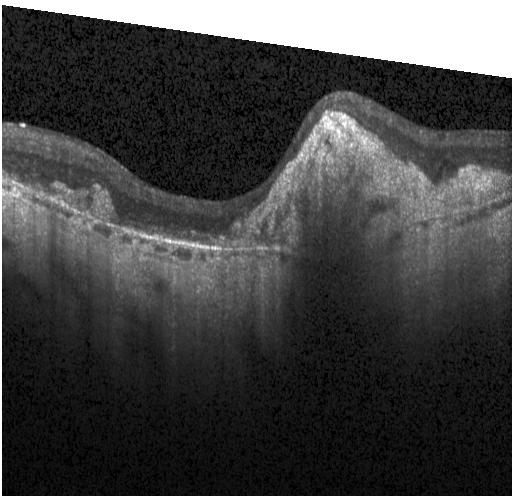 Spectral-domain optical coherence tomography, macular scan, optical coherence tomography scan, Heidelberg Spectralis. Dx: CNV.